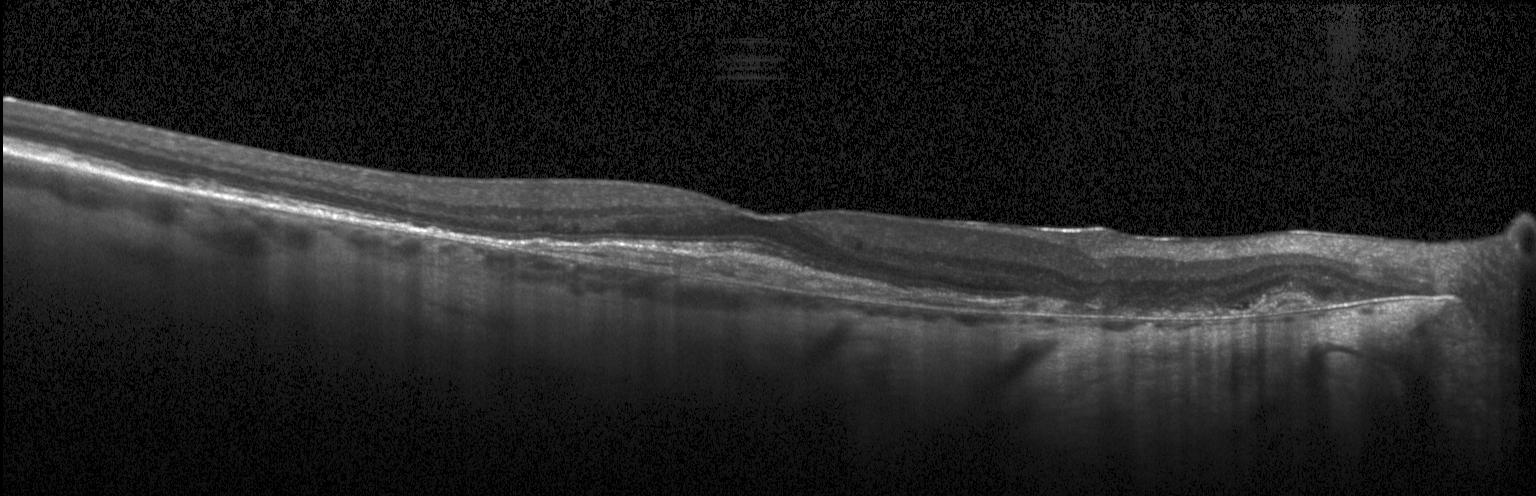

Optical coherence tomography scan.
This B-scan demonstrates a choroidal neovascular membrane.